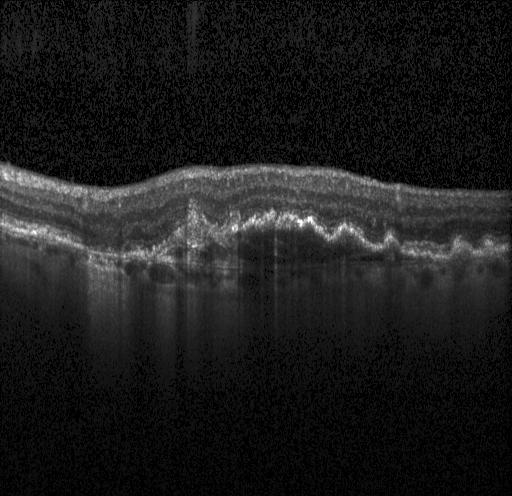

Optical coherence tomography scan · SD-OCT · Heidelberg Spectralis · macular scan — Dx: CNV.